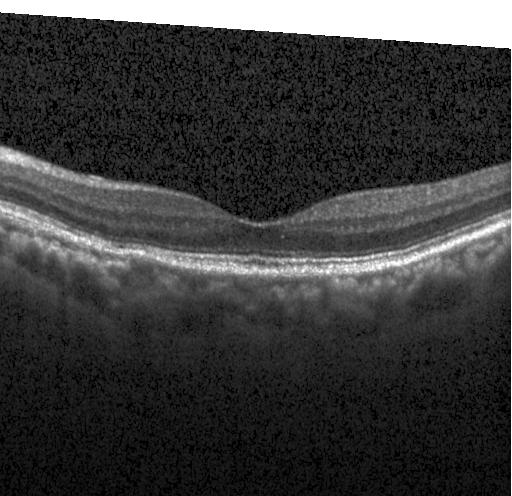 Assessment: no evidence of choroidal neovascularization, diabetic macular edema, or drusen.